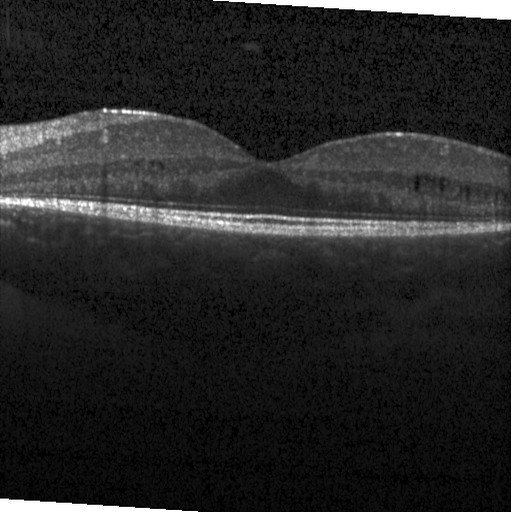
Macular OCT demonstrating DME.